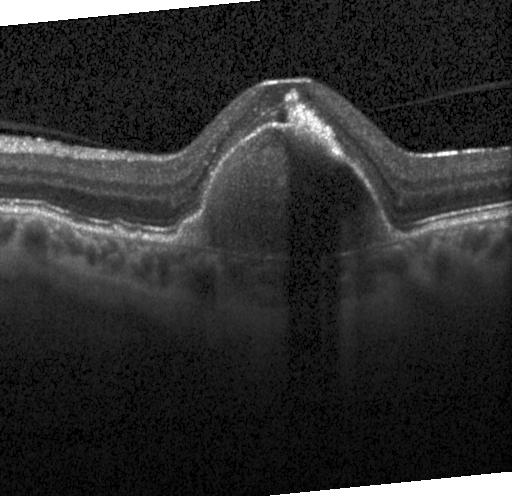 OCT B-scan · through the macula · SD-OCT
The scan shows choroidal neovascularization.